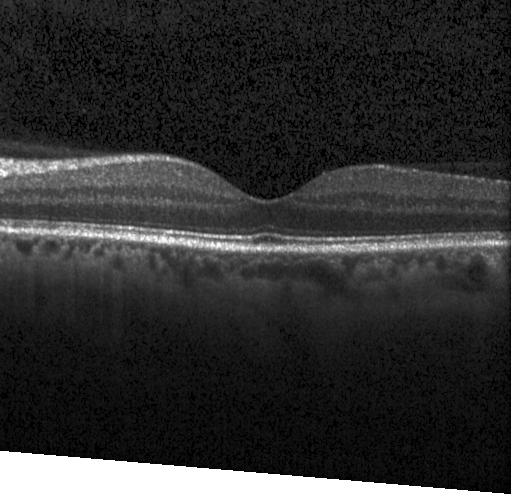

OCT line scan
Finding: no evidence of choroidal neovascularization, diabetic macular edema, or drusen.